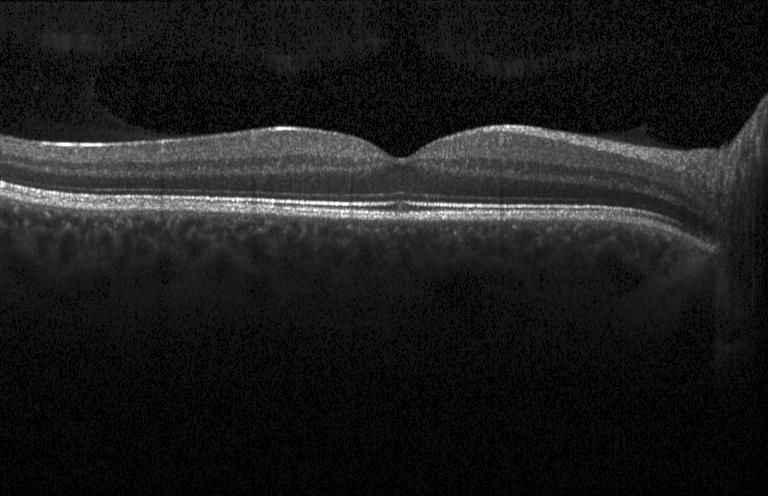

SD-OCT. Heidelberg Spectralis OCT system. OCT B-scan. Finding: no evidence of choroidal neovascularization, diabetic macular edema, or drusen.